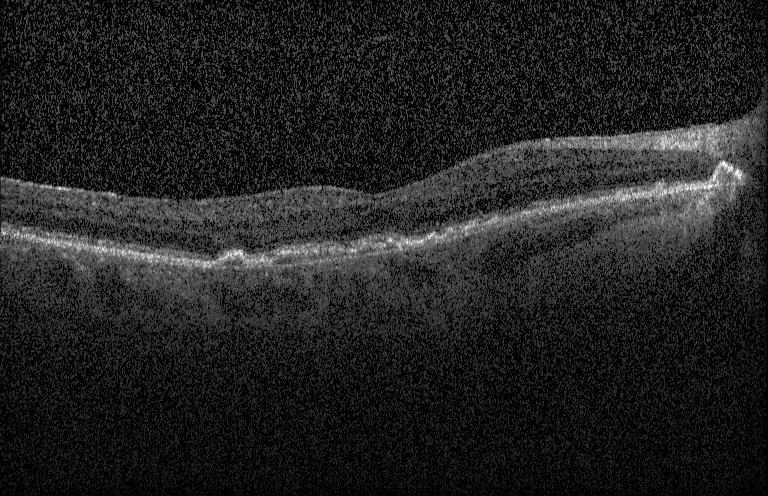
Diagnosis: a choroidal neovascular membrane.